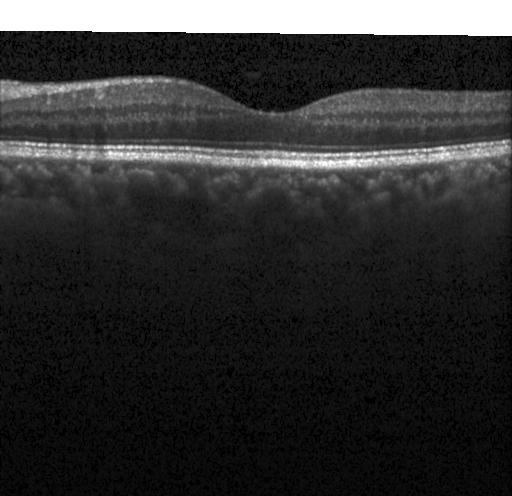 Retinal OCT cross-section — Macular OCT: no choroidal neovascularization, no diabetic macular edema, and no drusen.